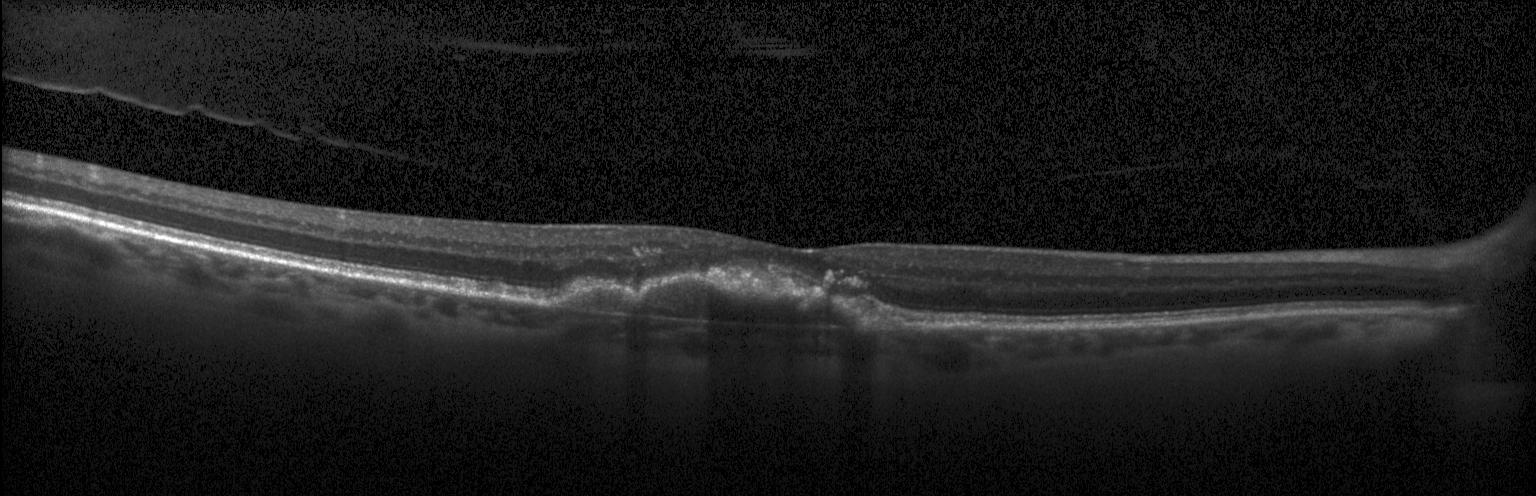

Finding: choroidal neovascularization.